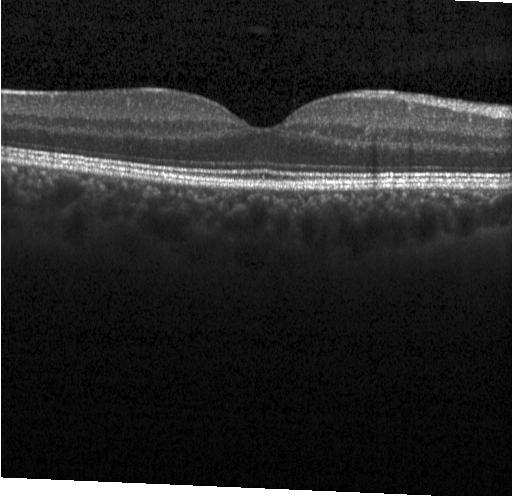 Horizontal scan through the fovea. Optical coherence tomography B-scan — This B-scan demonstrates no CNV, DME, or drusen.